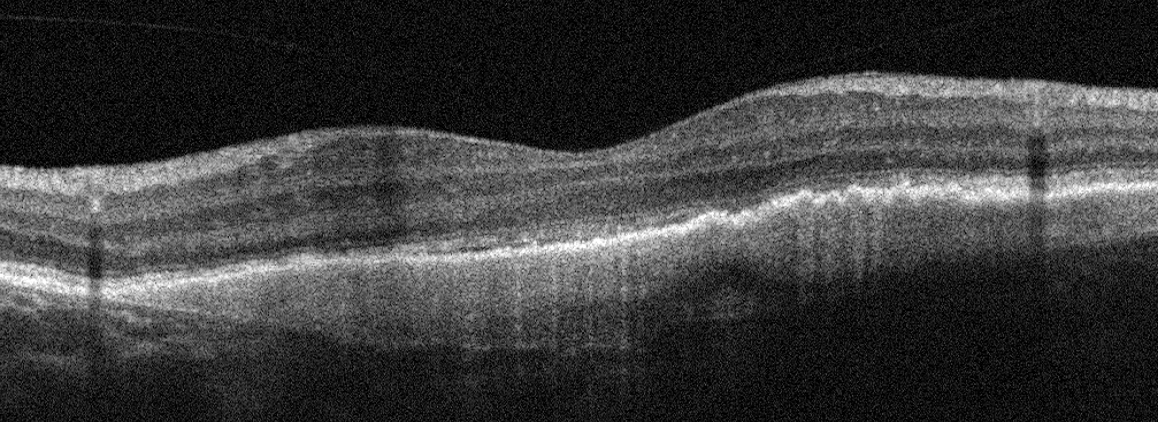 Instrument: Optovue Avanti RTVue XR; left eye; retinal OCT B-scan; through the macula — Assessment: AMD.